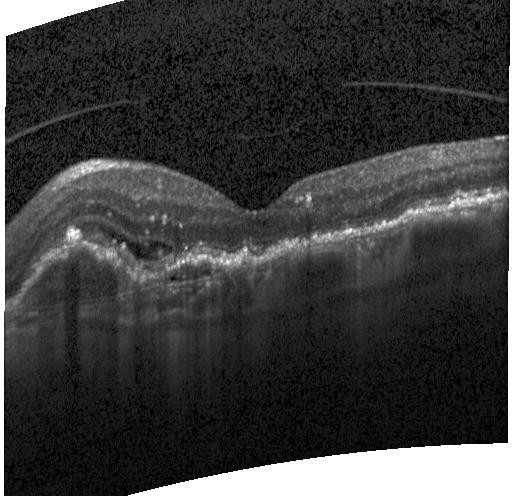
Acquired on a Heidelberg Spectralis · spectral-domain optical coherence tomography · horizontal scan through the fovea · OCT line scan. This B-scan demonstrates a choroidal neovascular membrane.